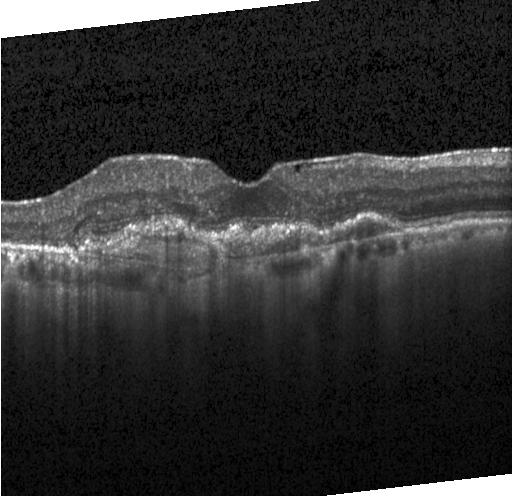 Macular OCT: CNV.